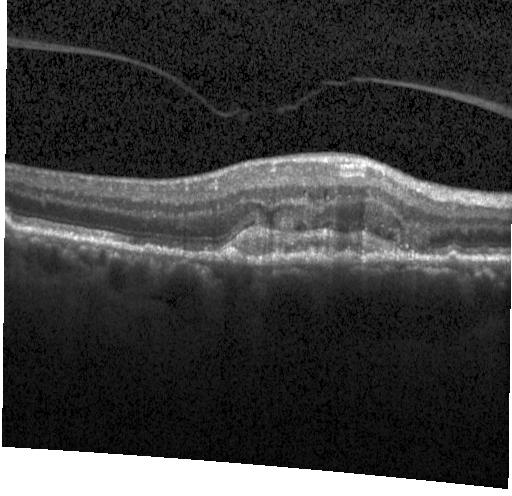 Instrument: Heidelberg Spectralis · retinal OCT B-scan · SD-OCT
Finding: CNV.